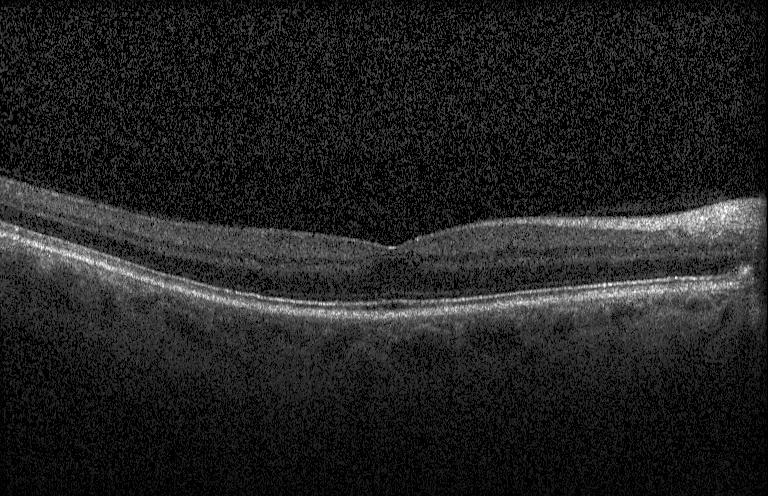
OCT line scan · Heidelberg Spectralis · spectral-domain OCT
This B-scan demonstrates no evidence of choroidal neovascularization, diabetic macular edema, or drusen.